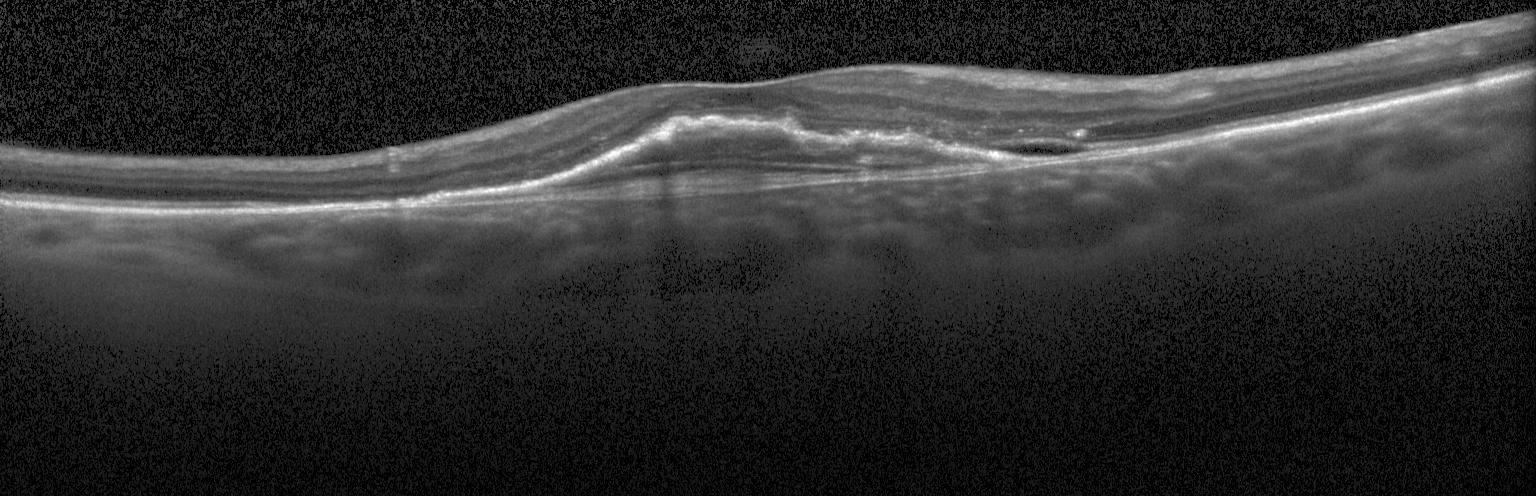

Assessment: a choroidal neovascular membrane.